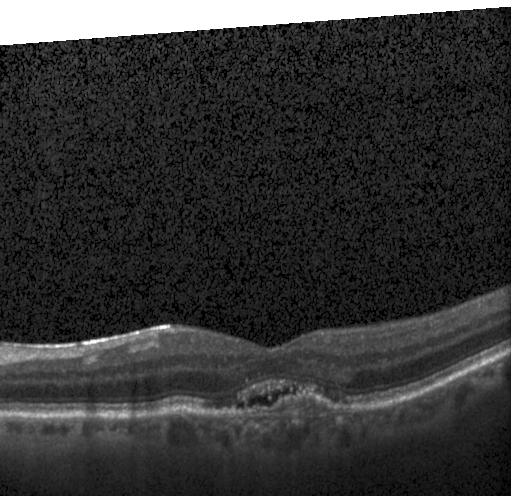
Choroidal neovascularization.